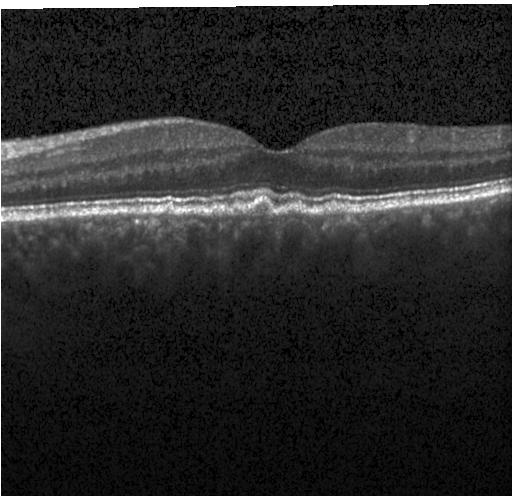

Diagnosis: sub-RPE drusenoid deposits.